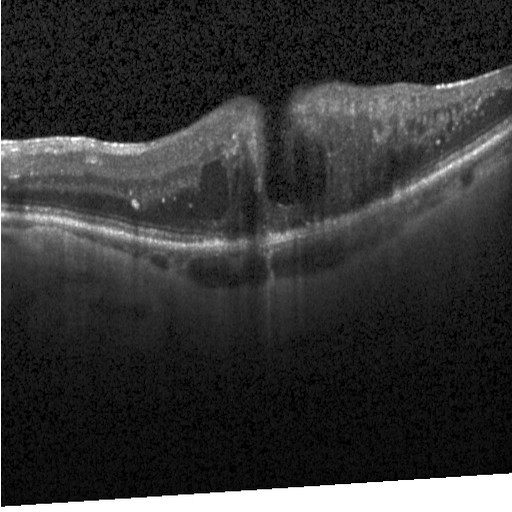

Spectral-domain OCT; optical coherence tomography scan — Assessment: diabetic macular edema (DME).